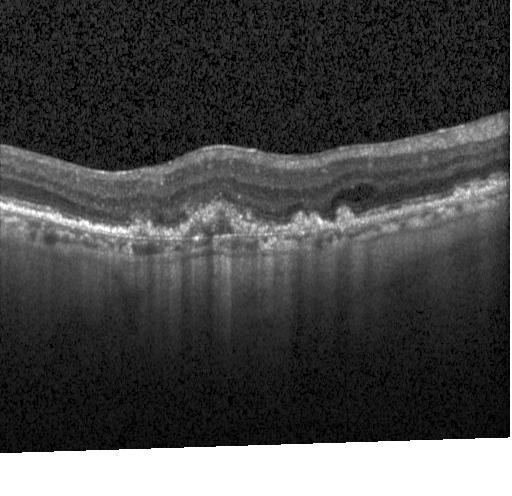 Acquired on a Heidelberg Spectralis; retinal OCT B-scan. Diagnosis: CNV.